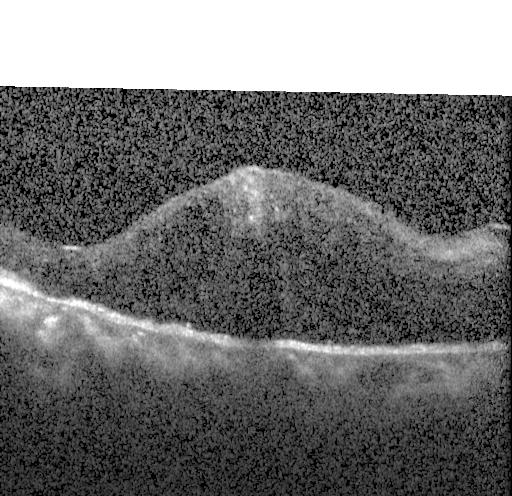 OCT B-scan.
Finding: DME.